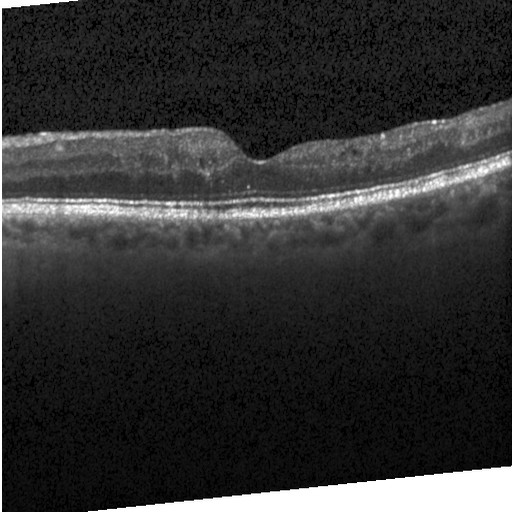 OCT line scan · acquired on a Heidelberg Spectralis. Impression: DME.